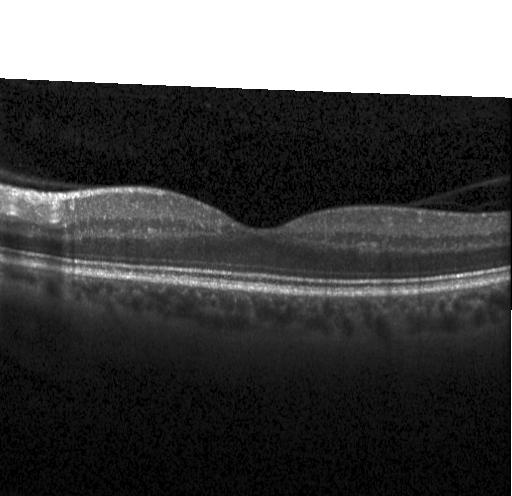

Dx: no choroidal neovascularization, no diabetic macular edema, and no drusen.